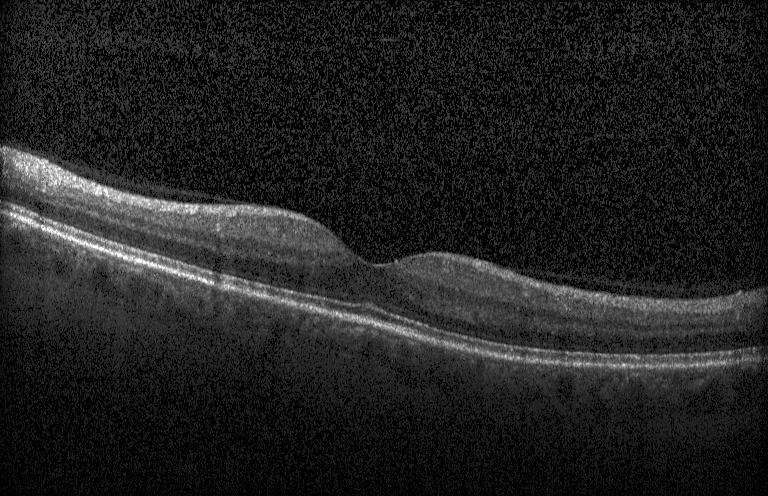
Diagnosis: neither CNV, DME, nor drusen.